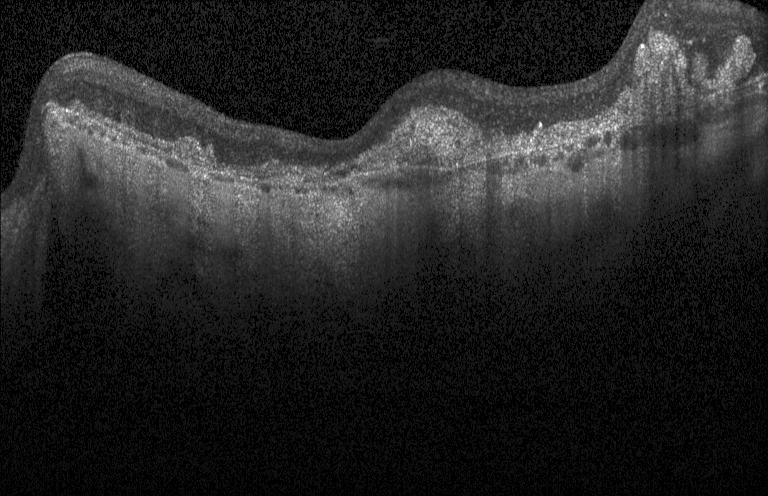
Dx: a choroidal neovascular membrane.